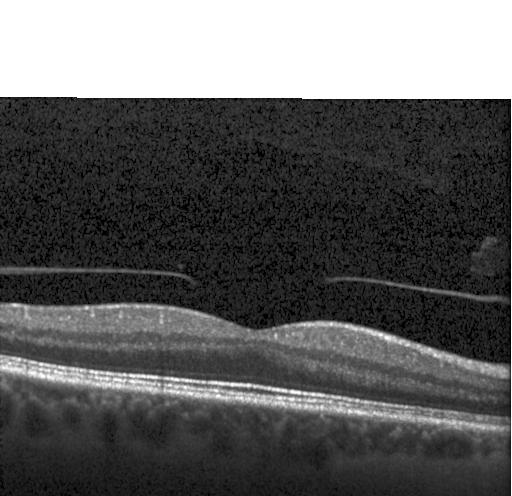
Instrument: Heidelberg Spectralis; centered on the fovea; OCT line scan; SD-OCT. Macular OCT: neither CNV, DME, nor drusen.